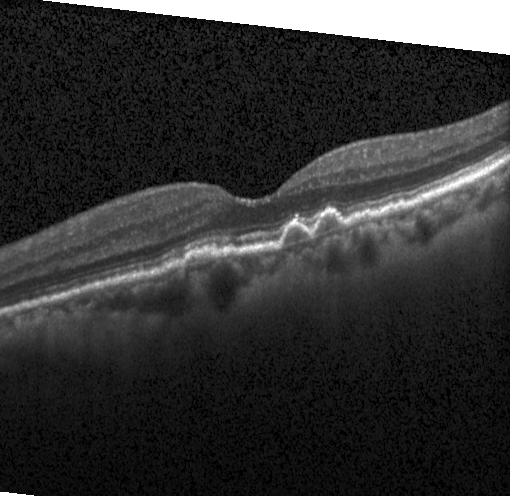 Retinal OCT cross-section — Assessment: multiple drusen.